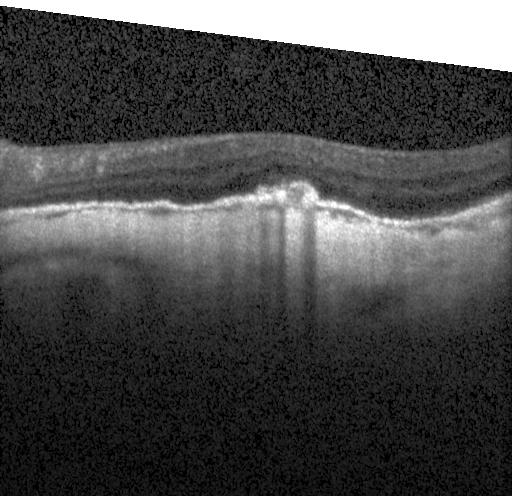
Retinal OCT B-scan; Heidelberg Spectralis OCT system.
The scan shows CNV.